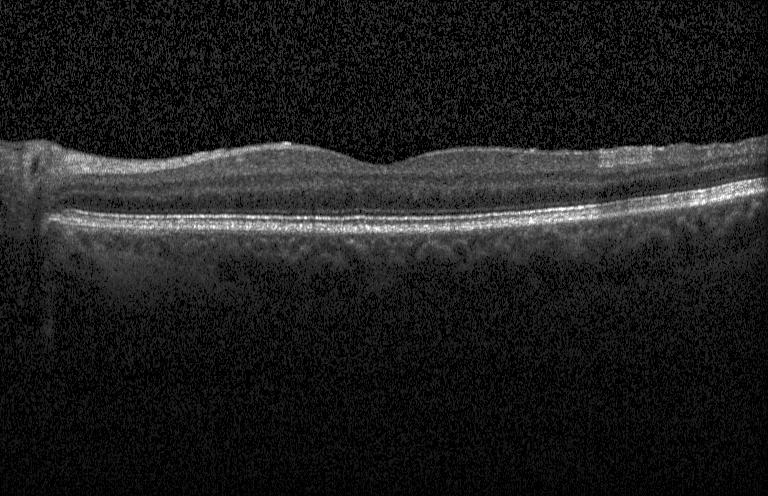

Optical coherence tomography scan. Centered on the fovea. Spectral-domain OCT. Heidelberg Spectralis OCT system
Finding: no CNV, DME, or drusen.